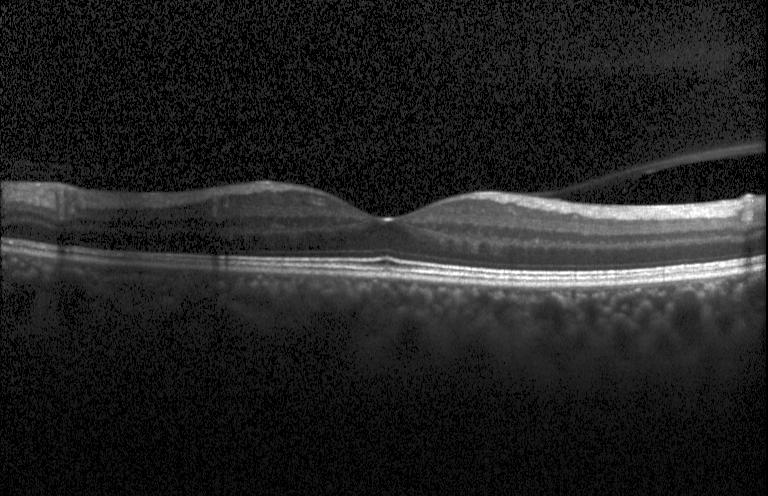 OCT finding: no choroidal neovascularization, no diabetic macular edema, and no drusen.